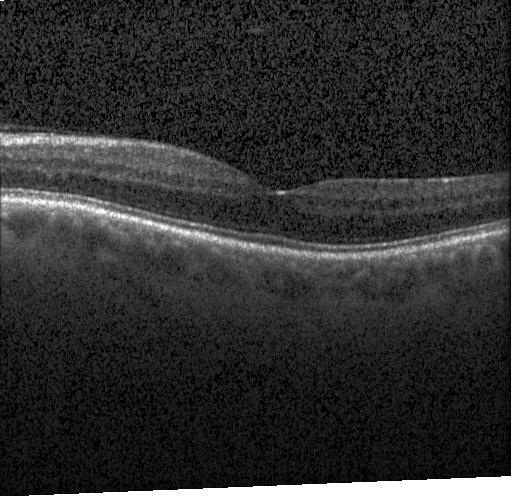
The scan shows no evidence of choroidal neovascularization, diabetic macular edema, or drusen.